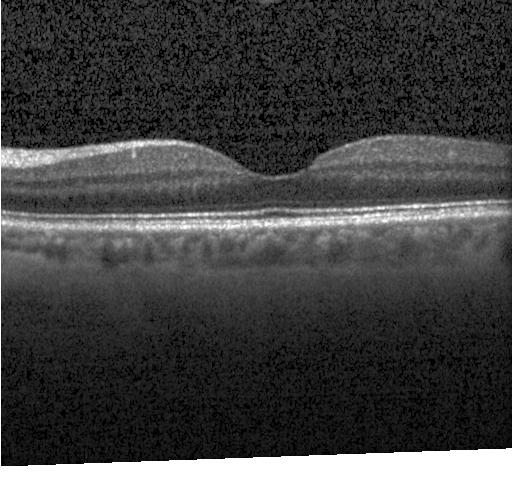 Horizontal scan through the fovea · retinal OCT B-scan
This B-scan demonstrates no CNV, DME, or drusen.